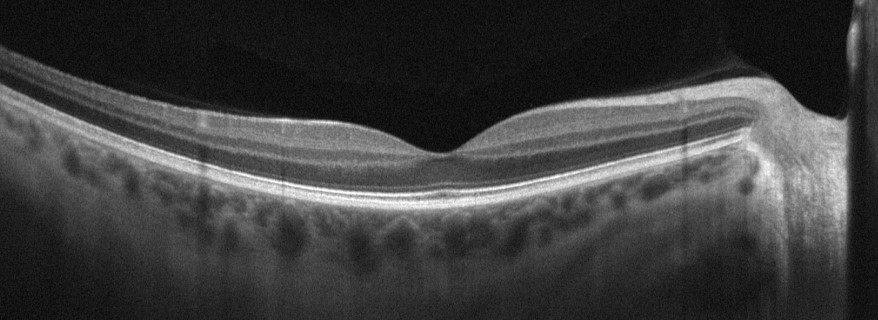
Impression: absence of AMD, DME, ERM, RAO, RVO, and vitreomacular interface disease.